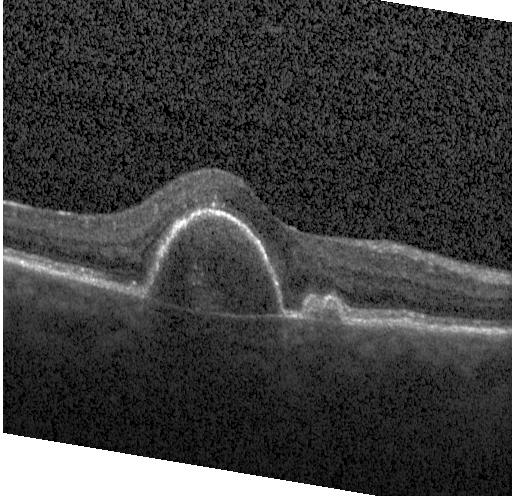 Diagnosis: a choroidal neovascular membrane.